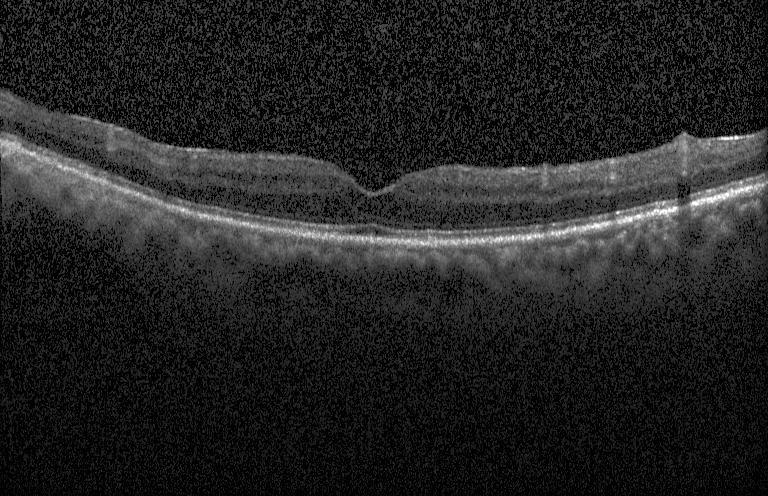

OCT B-scan; SD-OCT. Impression: no evidence of CNV, DME, or drusen.